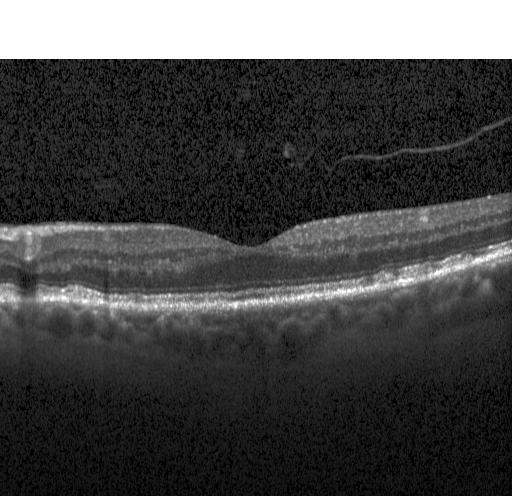
Acquired on a Heidelberg Spectralis, macular scan, OCT line scan, spectral-domain optical coherence tomography.
Impression: multiple drusen.